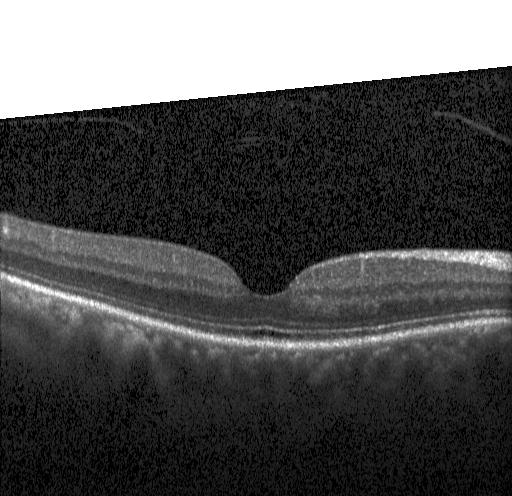 OCT line scan. Instrument: Heidelberg Spectralis
Impression: no evidence of choroidal neovascularization, diabetic macular edema, or drusen.